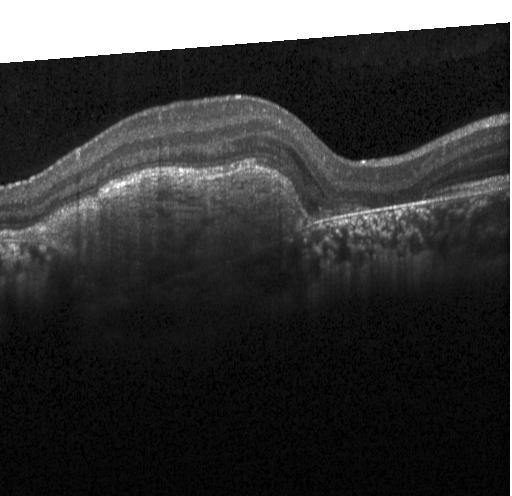
Centered on the fovea; spectral-domain optical coherence tomography; retinal OCT cross-section — Finding: choroidal neovascularization.